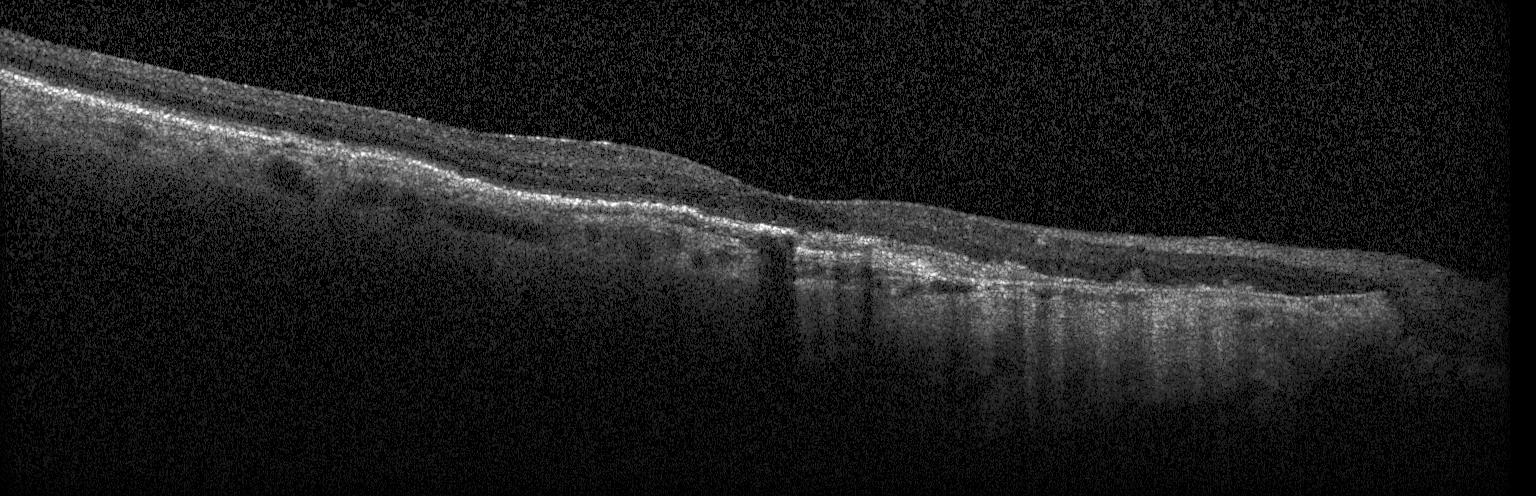
Spectral-domain OCT, retinal OCT B-scan. Dx: CNV.